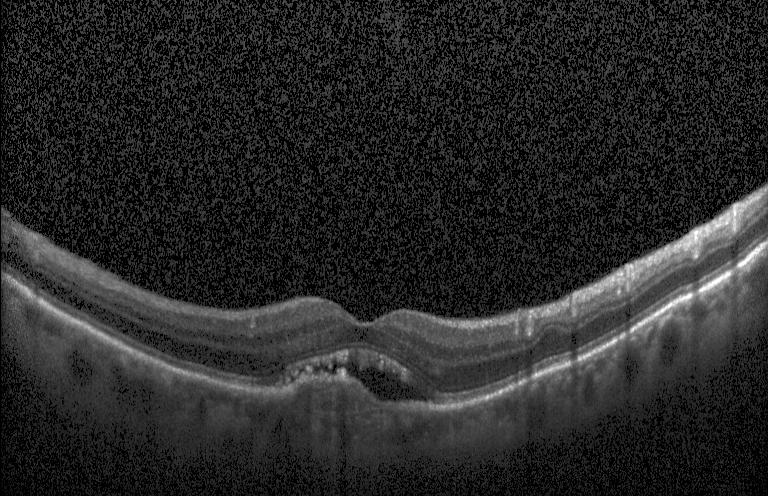 Heidelberg Spectralis; optical coherence tomography B-scan
Finding: a choroidal neovascular membrane.